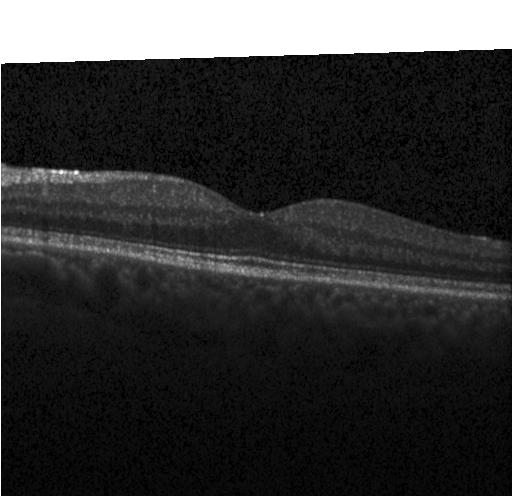 Retinal OCT cross-section.
The scan shows no choroidal neovascularization, diabetic macular edema, or drusen.